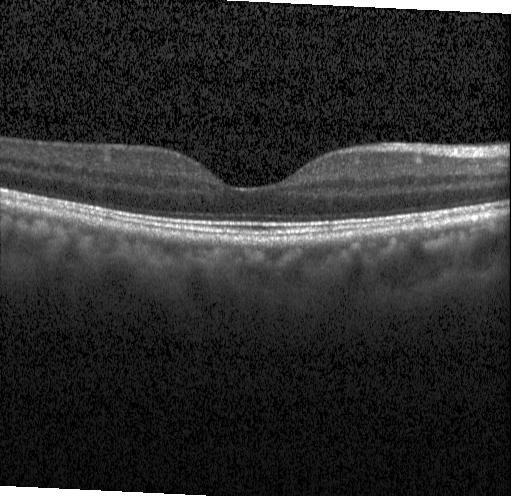 Macular OCT: no choroidal neovascularization, diabetic macular edema, or drusen.